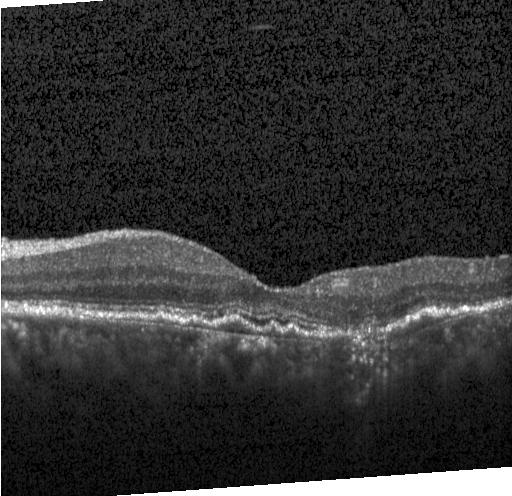

Macular OCT: a choroidal neovascular membrane.